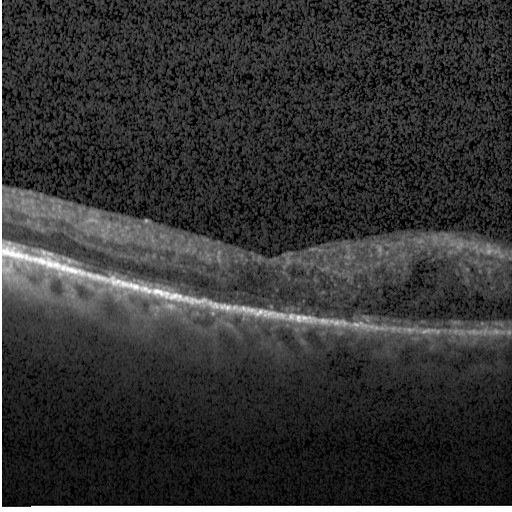 OCT line scan. DME.